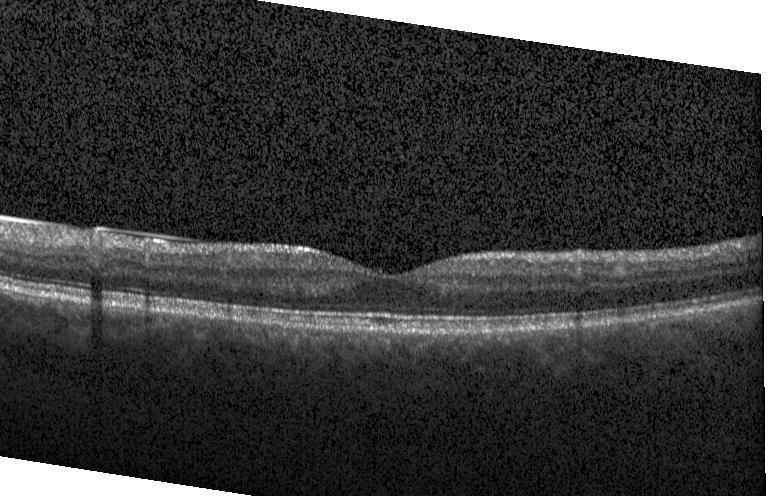

Spectral-domain OCT, optical coherence tomography scan
No evidence of choroidal neovascularization, diabetic macular edema, or drusen.